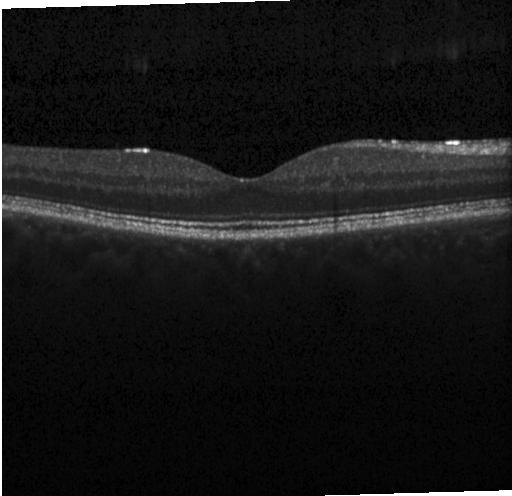

Spectral-domain OCT B-scan: no CNV, no DME, and no drusen.